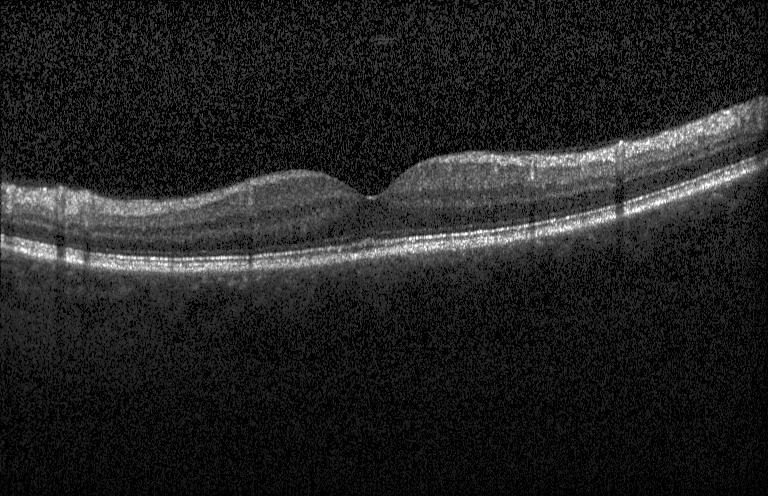
Impression: no choroidal neovascularization, diabetic macular edema, or drusen.